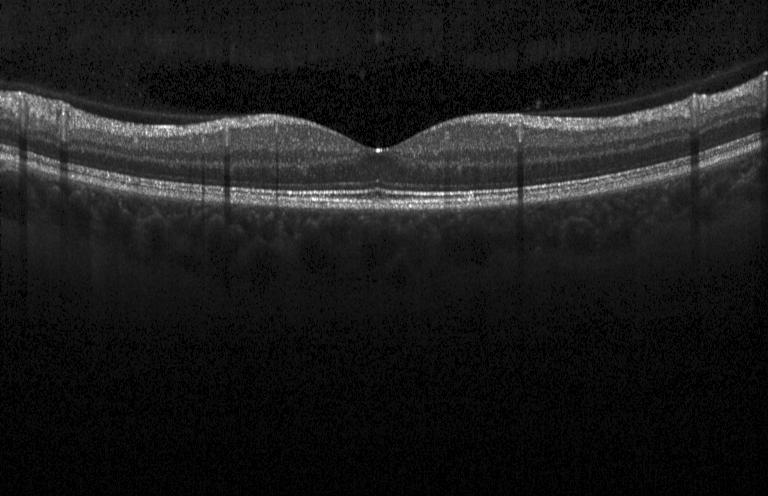
Finding: neither CNV, DME, nor drusen.